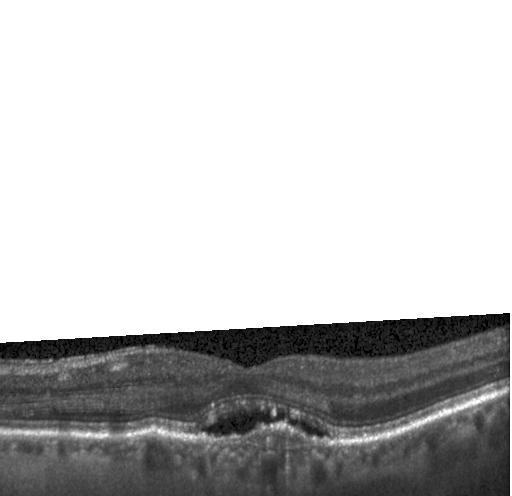 OCT line scan · Heidelberg Spectralis OCT system · SD-OCT — Assessment: choroidal neovascularization (CNV).